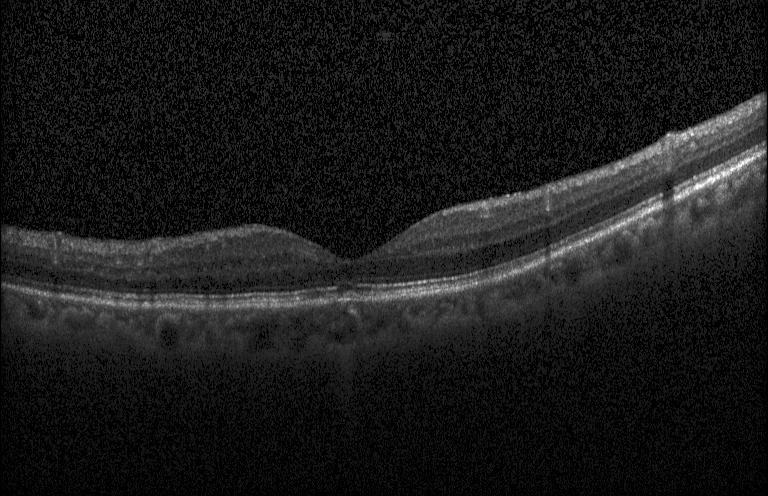
Instrument: Heidelberg Spectralis; retinal OCT B-scan; fovea-centered; spectral-domain OCT. OCT finding: no evidence of choroidal neovascularization, diabetic macular edema, or drusen.